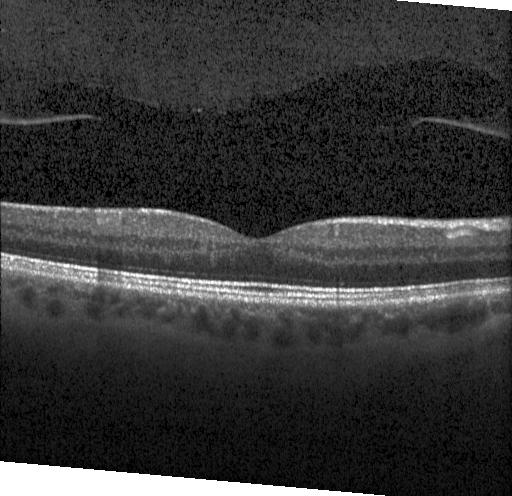 Optical coherence tomography scan
Diagnosis: no choroidal neovascularization, diabetic macular edema, or drusen.